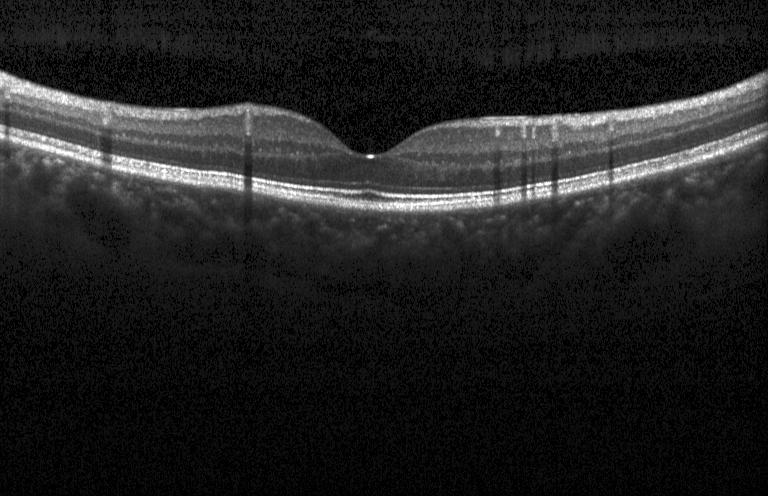

Spectral-domain OCT B-scan: no evidence of choroidal neovascularization, diabetic macular edema, or drusen.